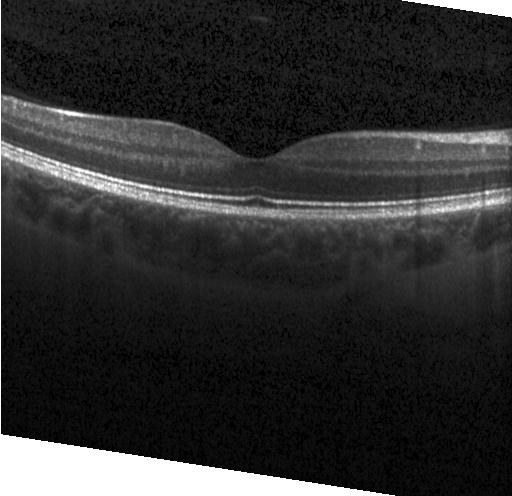
Impression: no CNV, no DME, and no drusen.